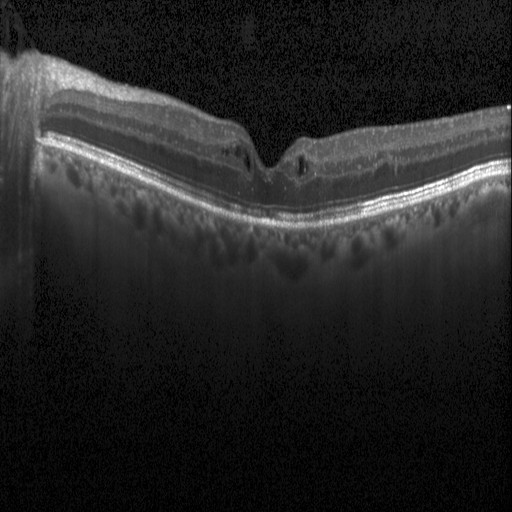
The scan shows DME.